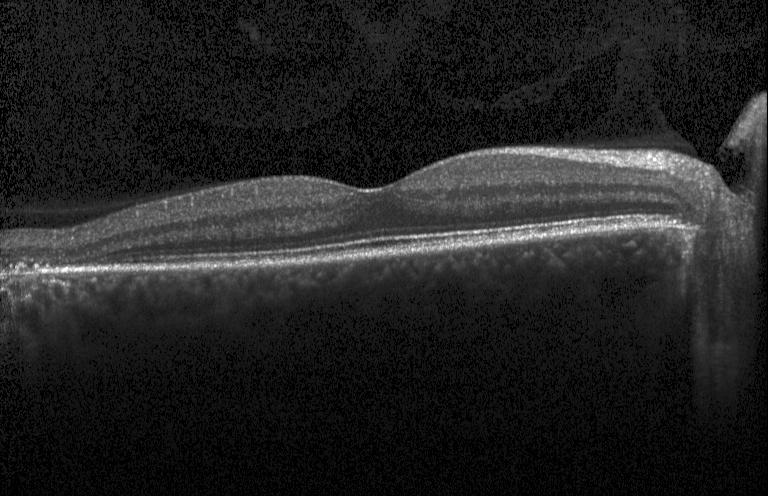 Retinal OCT B-scan.
Neither choroidal neovascularization, diabetic macular edema, nor drusen.